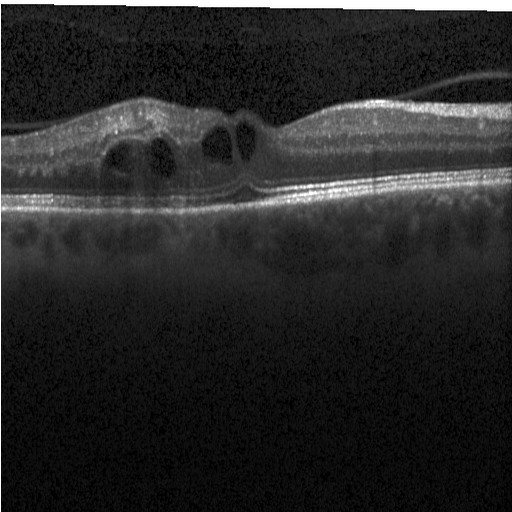 Optical coherence tomography B-scan, acquired on a Heidelberg Spectralis.
Finding: DME.